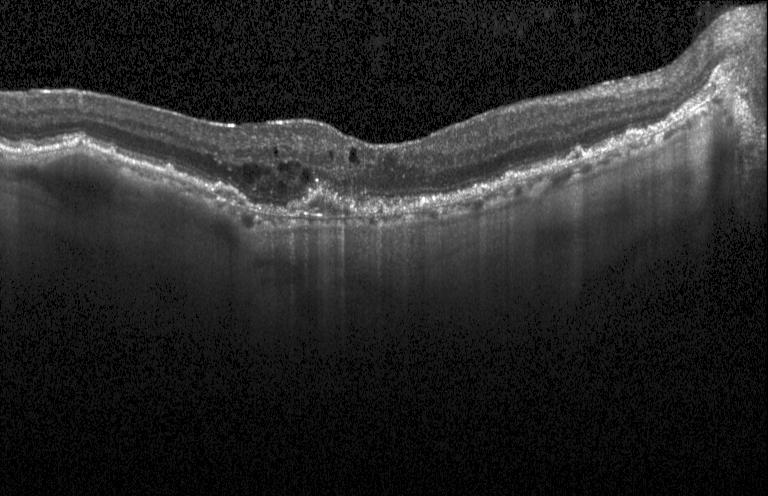 Finding: a choroidal neovascular membrane.